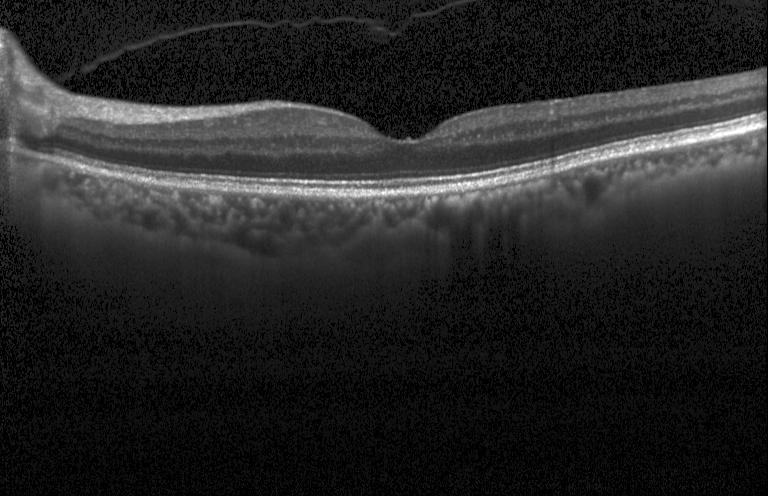

Optical coherence tomography scan
Assessment: neither choroidal neovascularization, diabetic macular edema, nor drusen.